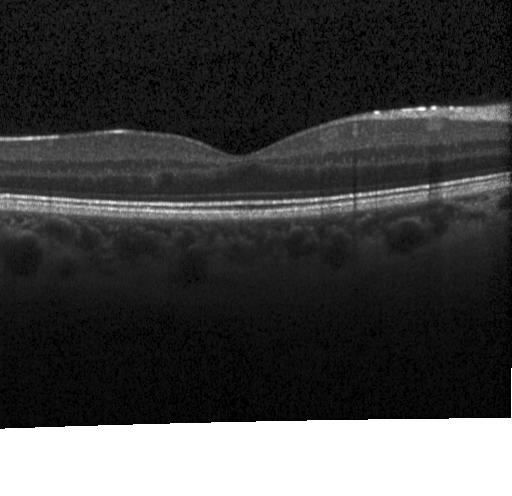

Optical coherence tomography B-scan. Spectral-domain optical coherence tomography. Macular scan. Impression: no evidence of choroidal neovascularization, diabetic macular edema, or drusen.